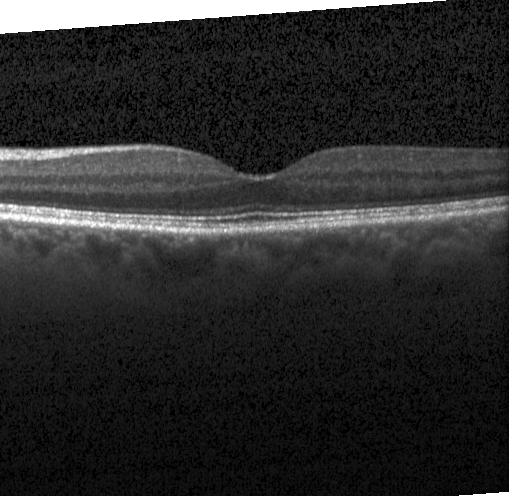
Acquired on a Heidelberg Spectralis; fovea-centered; retinal OCT B-scan — The scan shows no choroidal neovascularization, no diabetic macular edema, and no drusen.